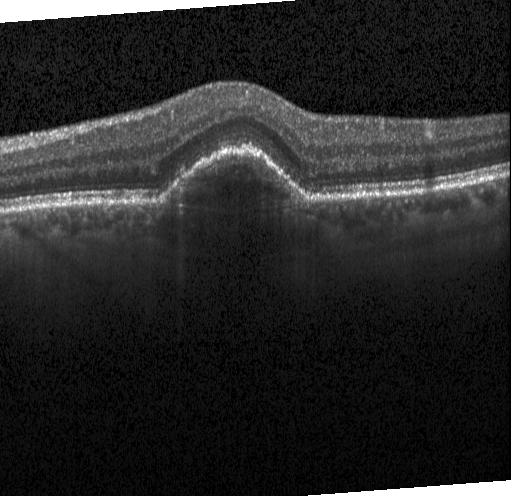

Spectral-domain OCT. Optical coherence tomography scan. Assessment: a choroidal neovascular membrane.